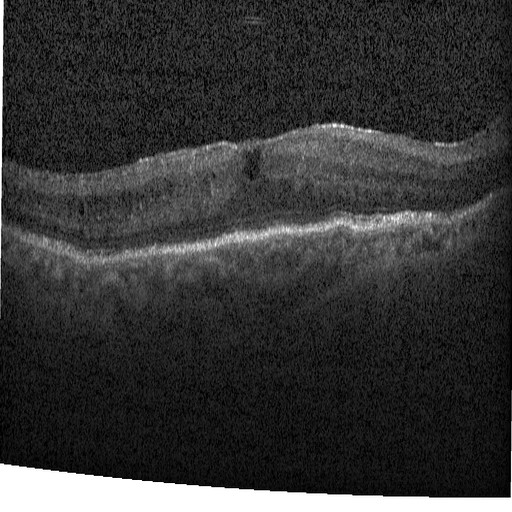 The scan shows diabetic macular edema (DME).